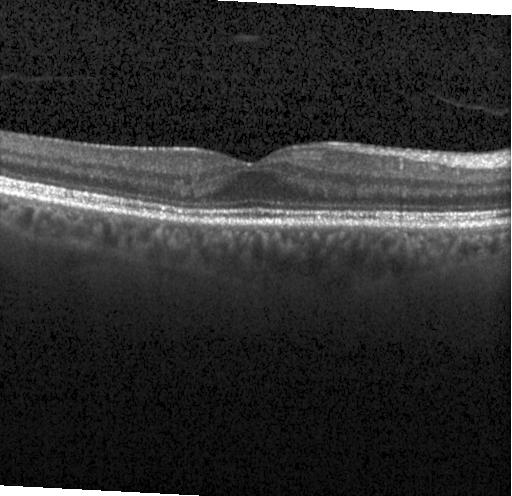 The scan shows neither choroidal neovascularization, diabetic macular edema, nor drusen.